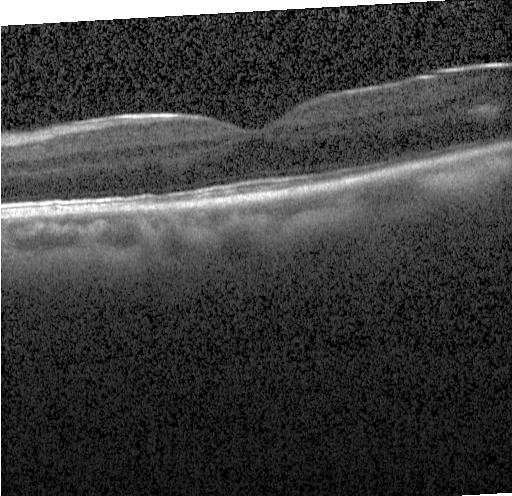
OCT B-scan.
Impression: no choroidal neovascularization, no diabetic macular edema, and no drusen.